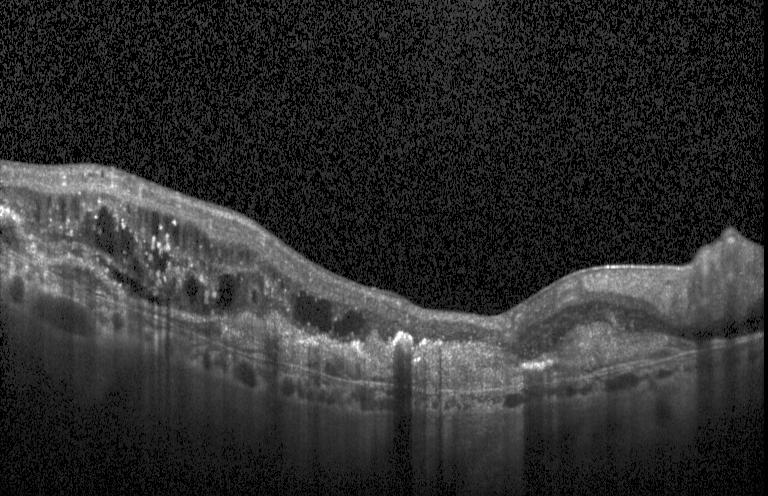
Diagnosis: choroidal neovascularization.